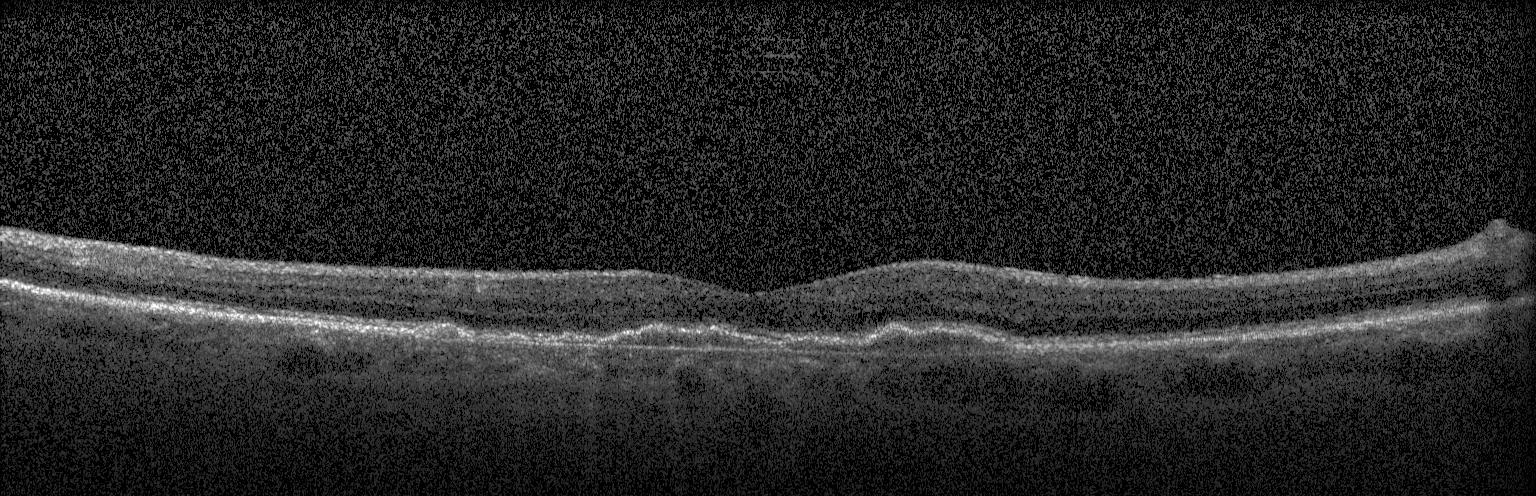 OCT scan showing choroidal neovascularization.